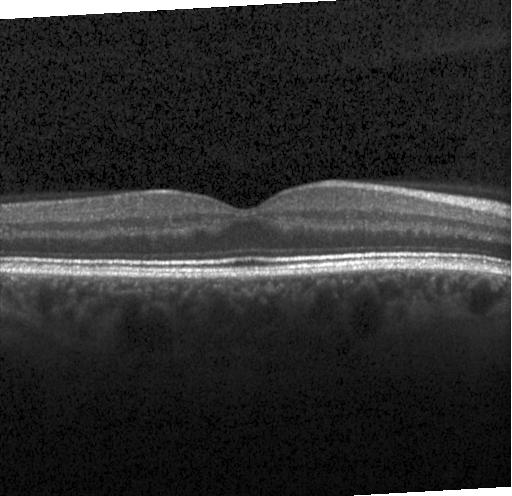 Assessment: neither CNV, DME, nor drusen.